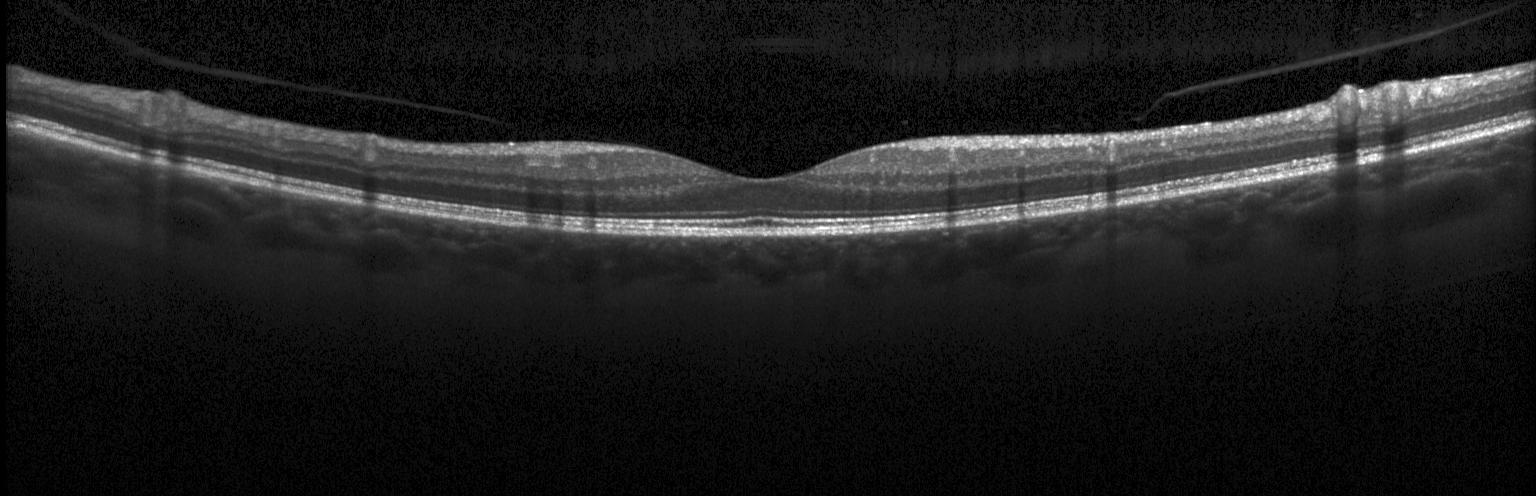

OCT line scan; centered on the fovea.
Finding: neither CNV, DME, nor drusen.